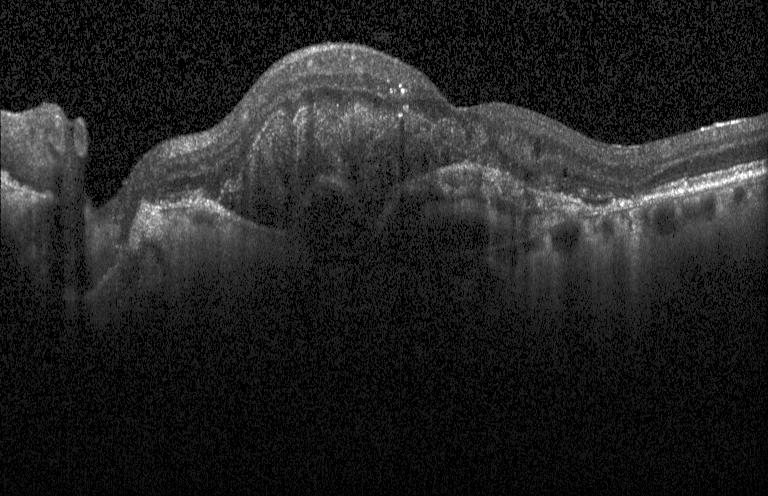

Spectral-domain OCT, instrument: Heidelberg Spectralis, retinal OCT B-scan, centered on the fovea.
The scan shows a choroidal neovascular membrane.